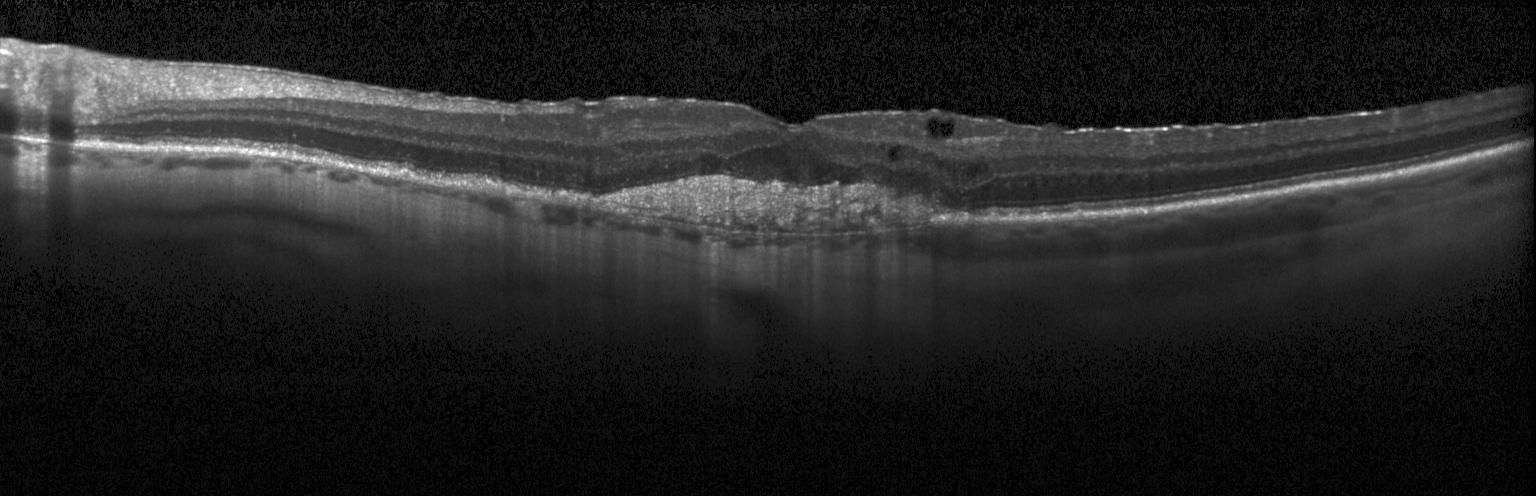 Centered on the fovea, SD-OCT, instrument: Heidelberg Spectralis, OCT B-scan.
The scan shows a choroidal neovascular membrane.